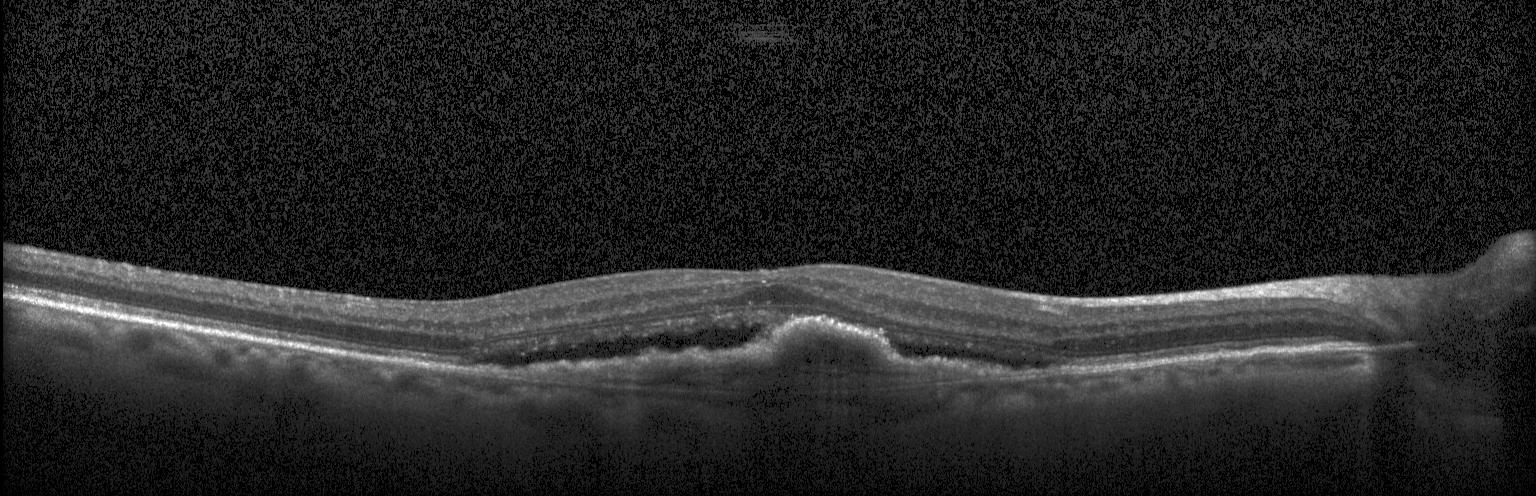 OCT finding: choroidal neovascularization.